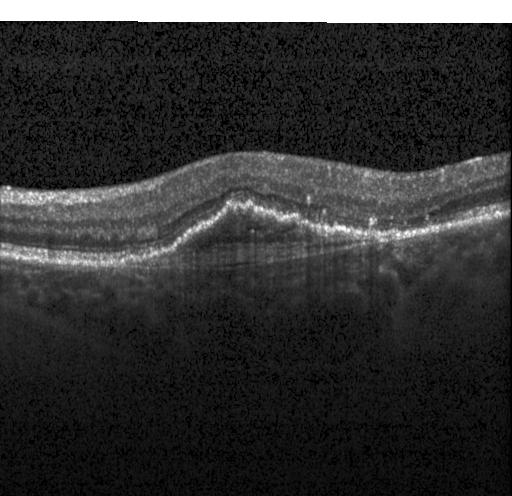 Spectral-domain OCT B-scan: choroidal neovascularization.